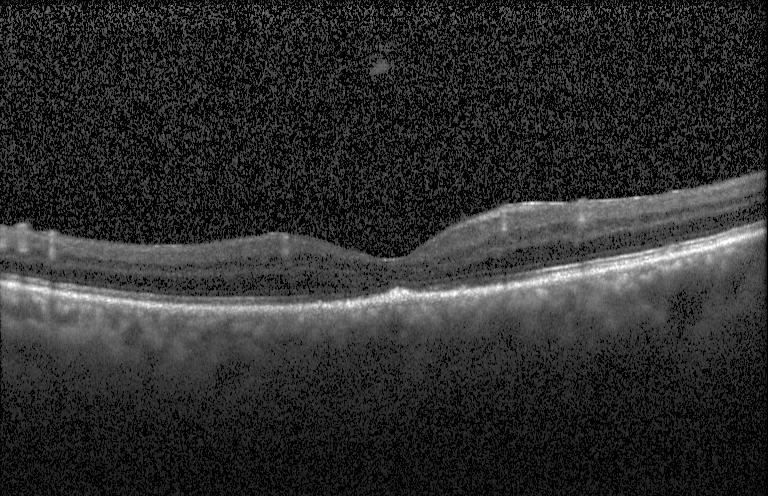 Spectral-domain OCT, centered on the fovea, optical coherence tomography scan, Heidelberg Spectralis OCT system. Assessment: sub-RPE drusenoid deposits.